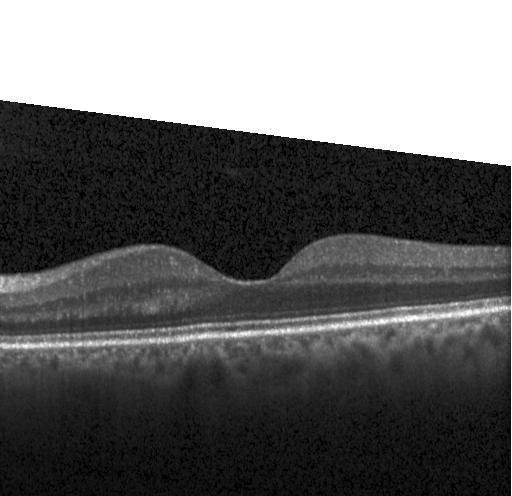
Retinal OCT B-scan, Heidelberg Spectralis OCT system, centered on the fovea, spectral-domain OCT. OCT finding: neither choroidal neovascularization, diabetic macular edema, nor drusen.